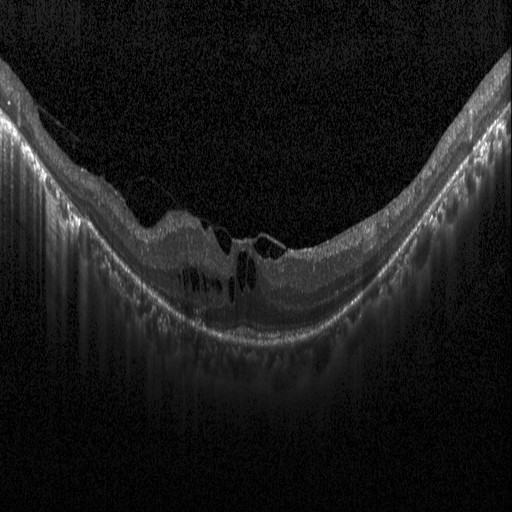

Heidelberg Spectralis. OCT B-scan
Macular OCT: DME.